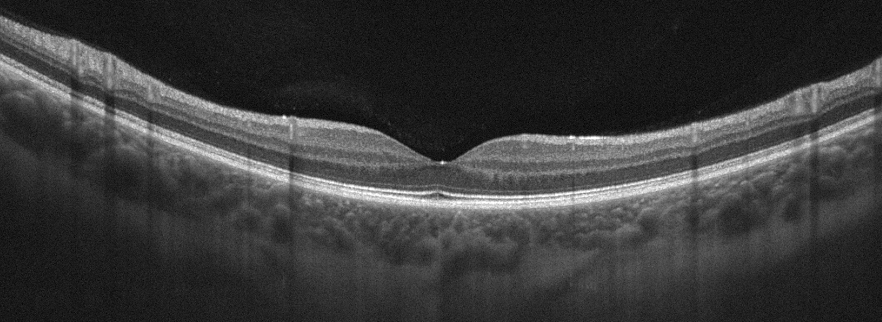
Retinal OCT cross-section showing absence of AMD, DME, ERM, RAO, RVO, and vitreomacular interface disease.